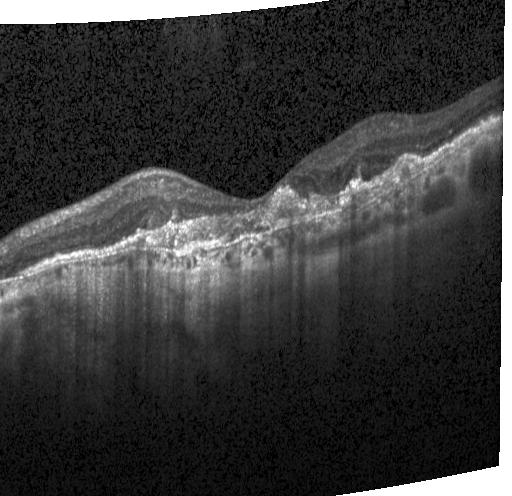
Macular OCT: a choroidal neovascular membrane.